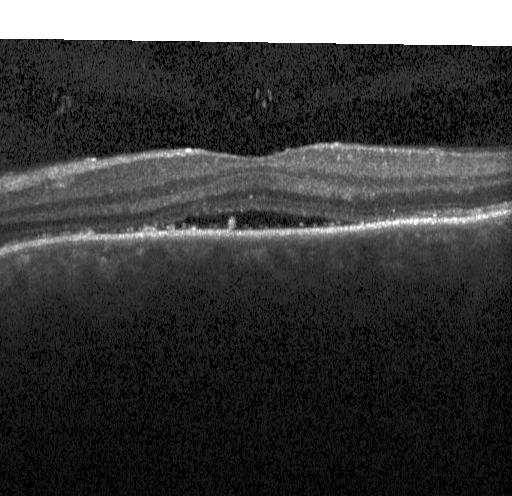

Retinal OCT cross-section. Finding: CNV.